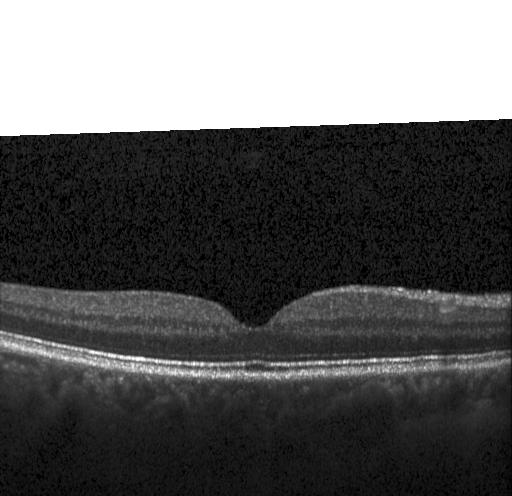

Finding: no evidence of CNV, DME, or drusen.